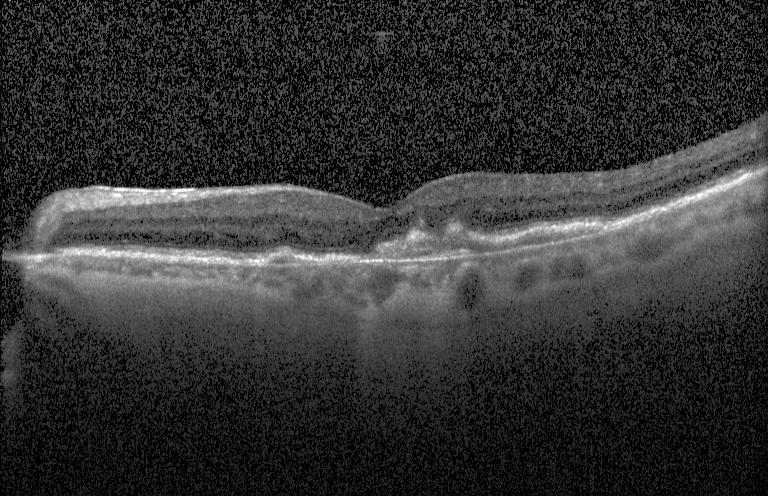

OCT finding: choroidal neovascularization.